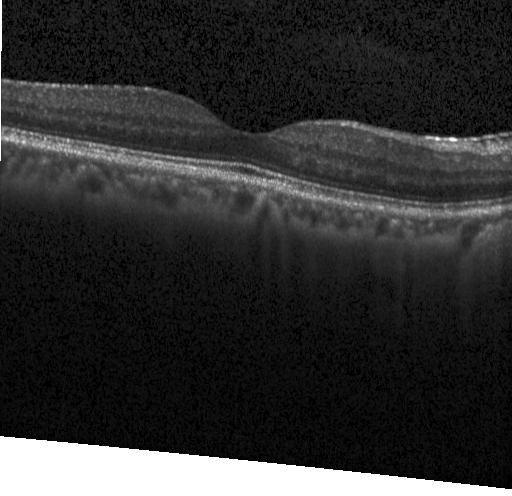

Fovea-centered · retinal OCT B-scan
Macular OCT: neither choroidal neovascularization, diabetic macular edema, nor drusen.